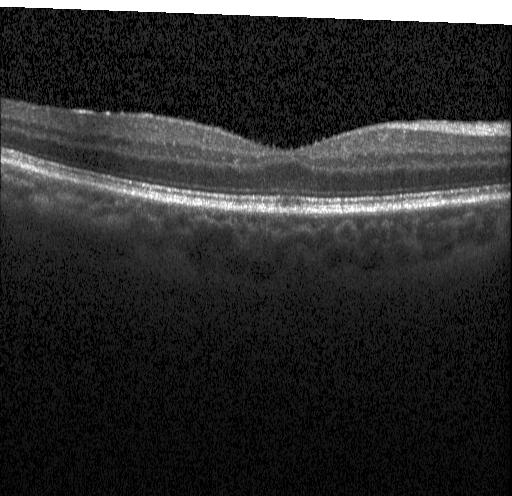
Assessment: no CNV, DME, or drusen.